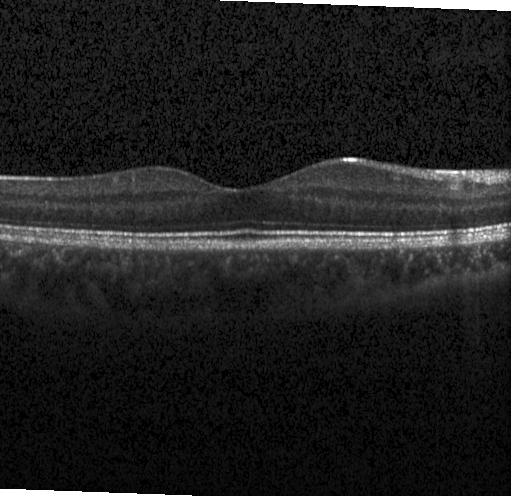
Retinal OCT cross-section. Impression: no evidence of choroidal neovascularization, diabetic macular edema, or drusen.